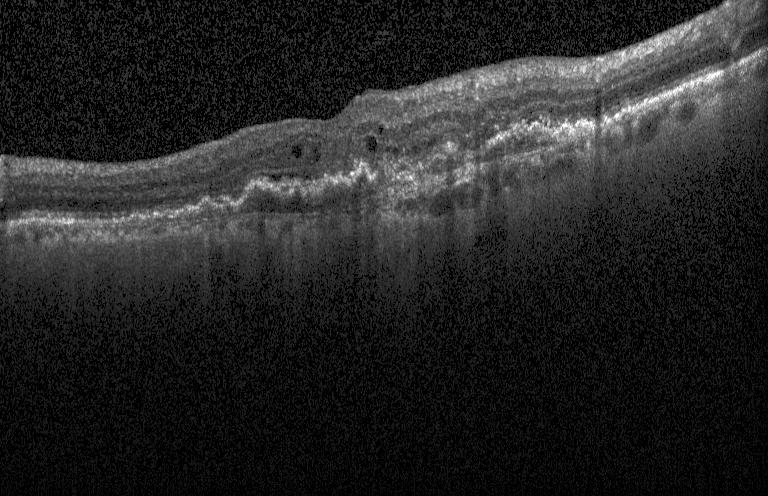
Through the macula; spectral-domain OCT; Heidelberg Spectralis; retinal OCT B-scan.
Diagnosis: choroidal neovascularization (CNV).